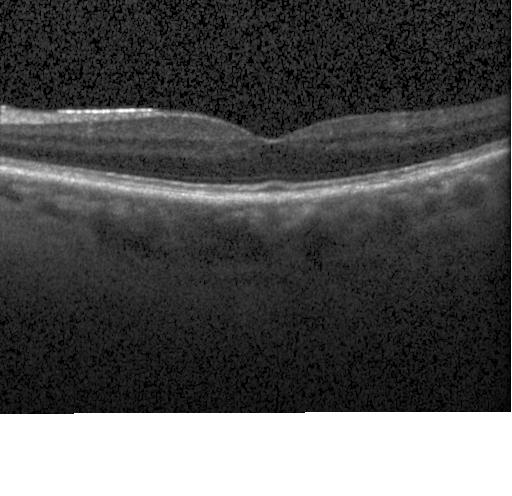

Heidelberg Spectralis OCT system. SD-OCT. Horizontal scan through the fovea. Optical coherence tomography B-scan
Diagnosis: neither choroidal neovascularization, diabetic macular edema, nor drusen.